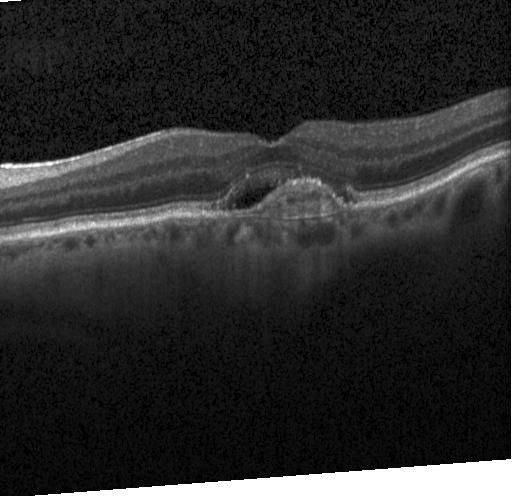

Retinal OCT cross-section showing a choroidal neovascular membrane.